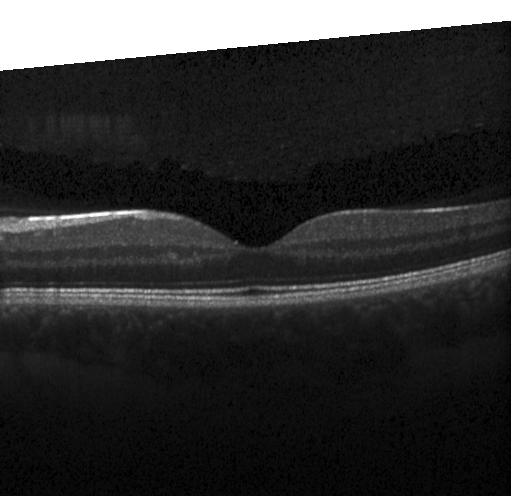

OCT finding: no evidence of choroidal neovascularization, diabetic macular edema, or drusen.